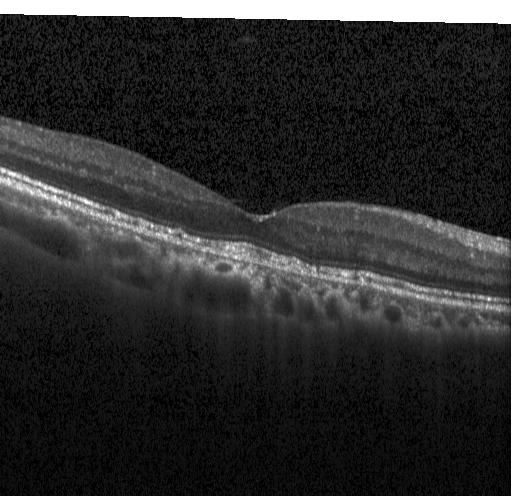
OCT B-scan — No evidence of choroidal neovascularization, diabetic macular edema, or drusen.